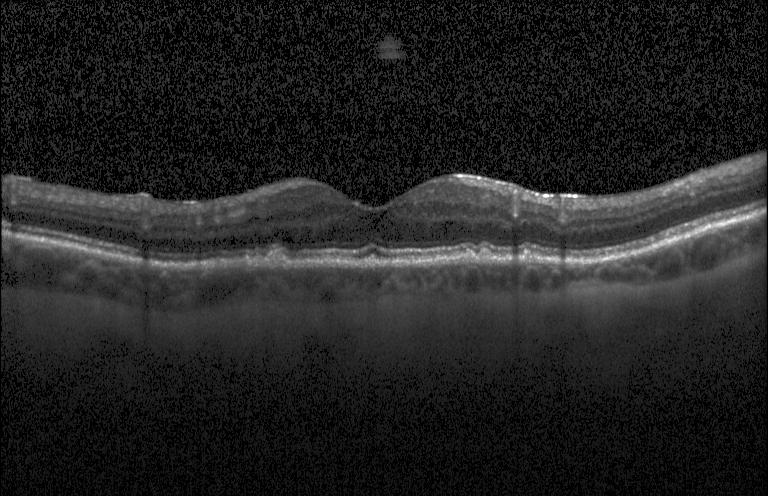

Through the macula; retinal OCT B-scan; acquired on a Heidelberg Spectralis; spectral-domain OCT — Assessment: drusen.